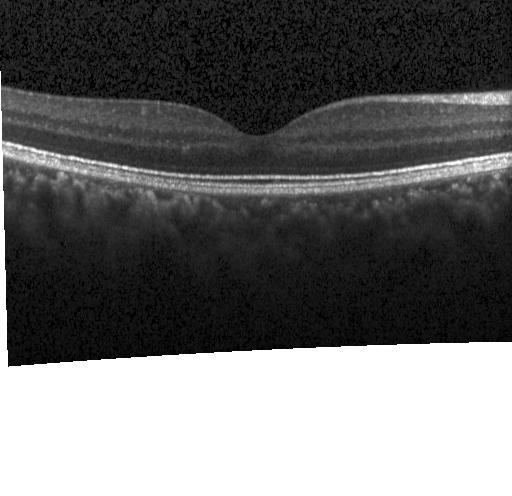
OCT line scan · spectral-domain optical coherence tomography. Diagnosis: no evidence of choroidal neovascularization, diabetic macular edema, or drusen.